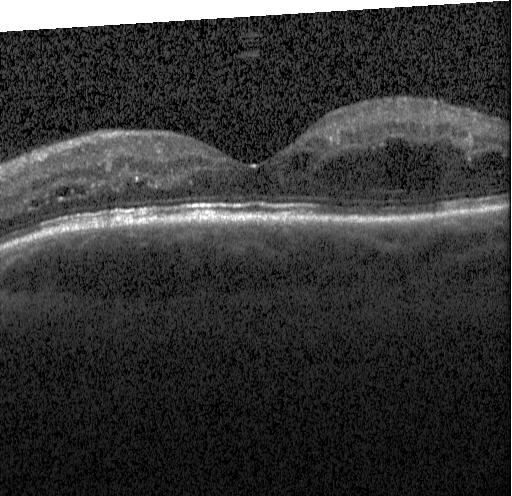 Assessment: diabetic macular edema.